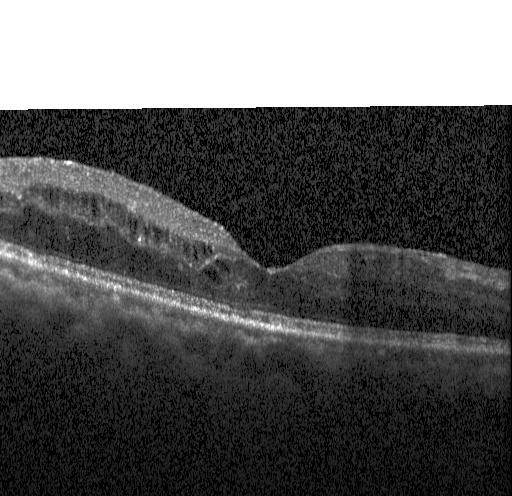 Retinal OCT cross-section
OCT finding: diabetic macular edema.